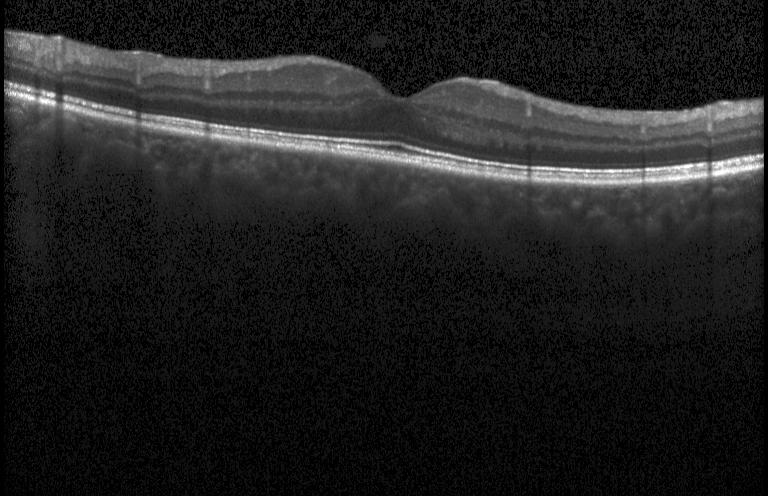 Heidelberg Spectralis OCT system; horizontal scan through the fovea; retinal OCT cross-section.
Macular OCT: no evidence of choroidal neovascularization, diabetic macular edema, or drusen.